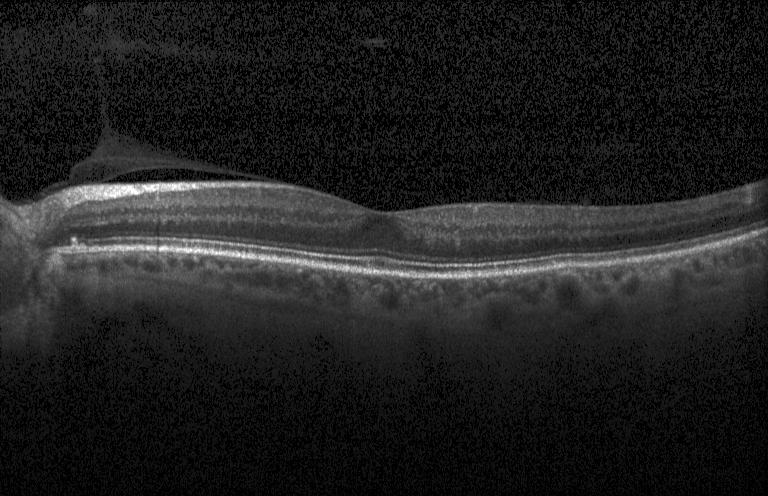

OCT finding: no evidence of choroidal neovascularization, diabetic macular edema, or drusen.